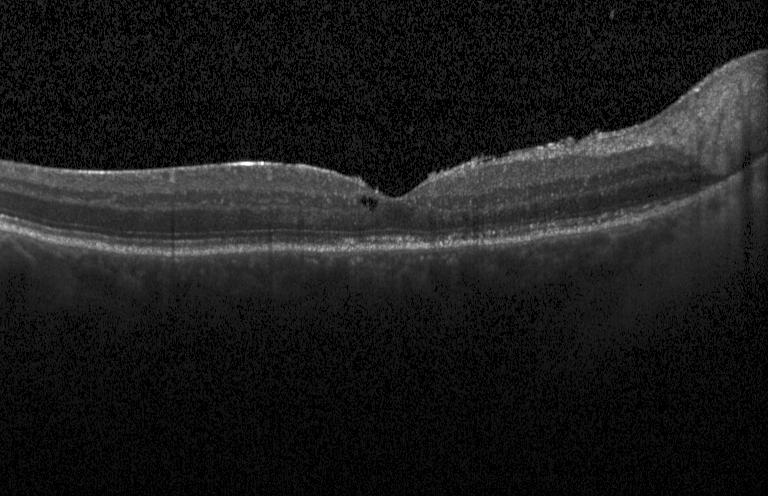

Optical coherence tomography B-scan, centered on the fovea, acquired on a Heidelberg Spectralis.
Diagnosis: DME.